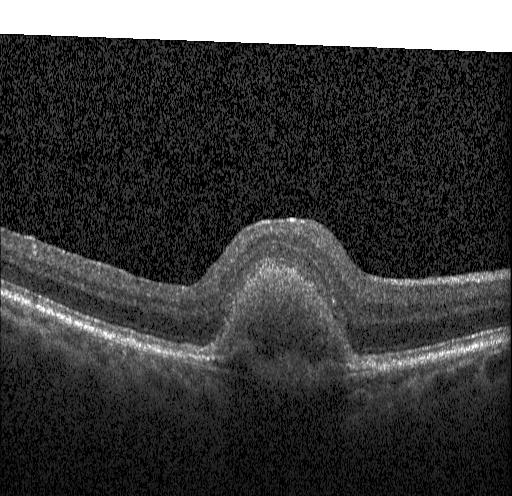
Dx: choroidal neovascularization.